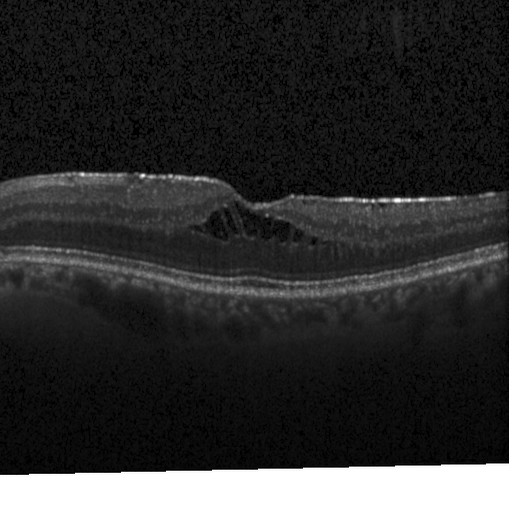
Optical coherence tomography scan; spectral-domain optical coherence tomography — Assessment: DME.